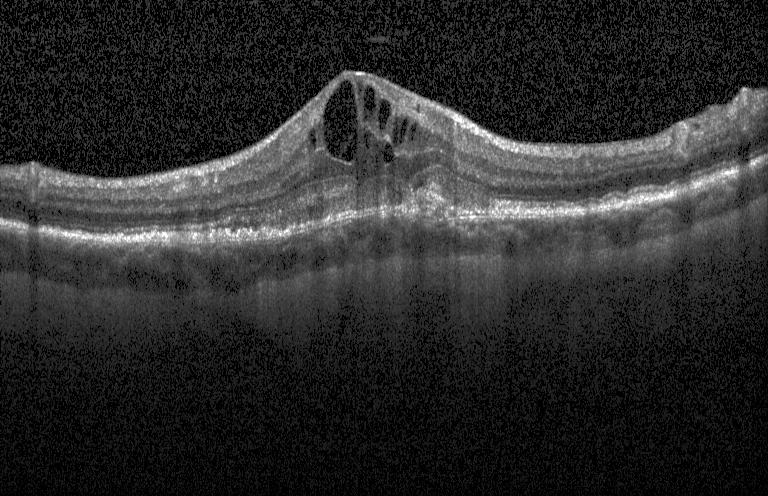

This B-scan demonstrates choroidal neovascularization (CNV).